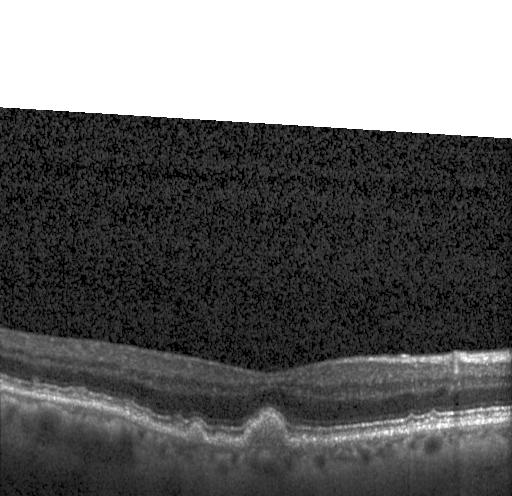 Retinal OCT B-scan
Diagnosis: multiple drusen.